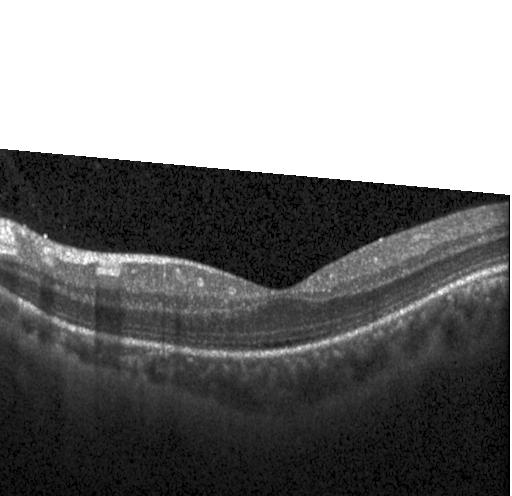 Fovea-centered; retinal OCT cross-section — OCT finding: no choroidal neovascularization, no diabetic macular edema, and no drusen.